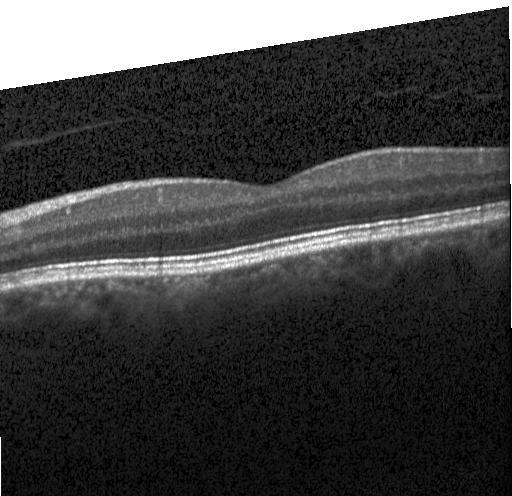
OCT finding: neither choroidal neovascularization, diabetic macular edema, nor drusen.